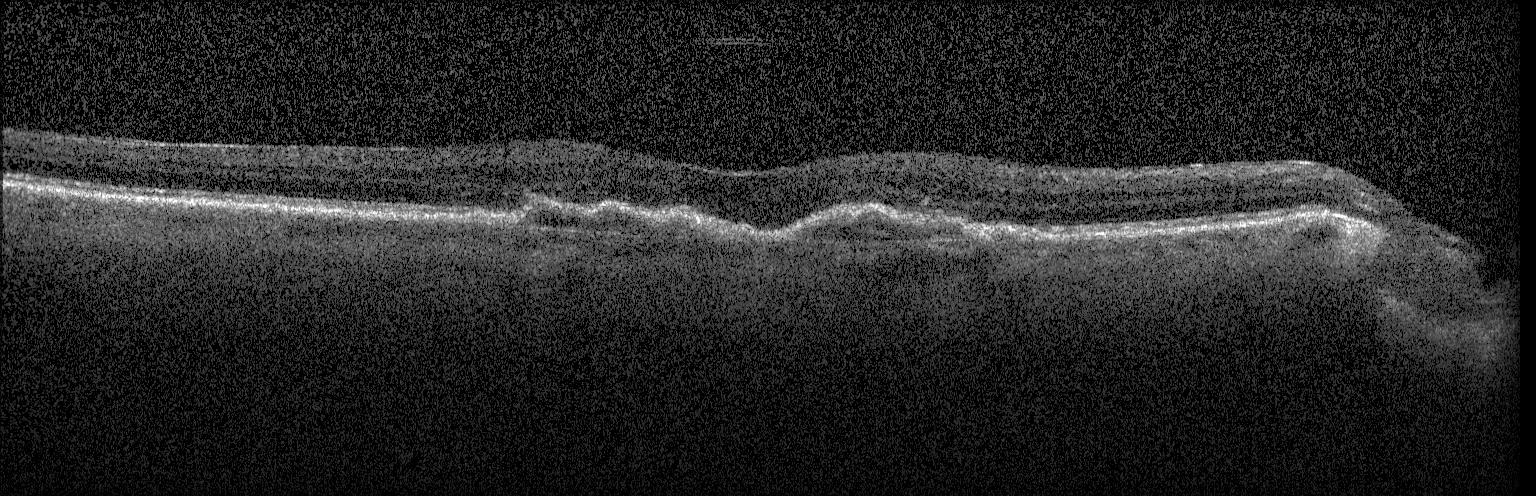
Retinal OCT cross-section showing a choroidal neovascular membrane.